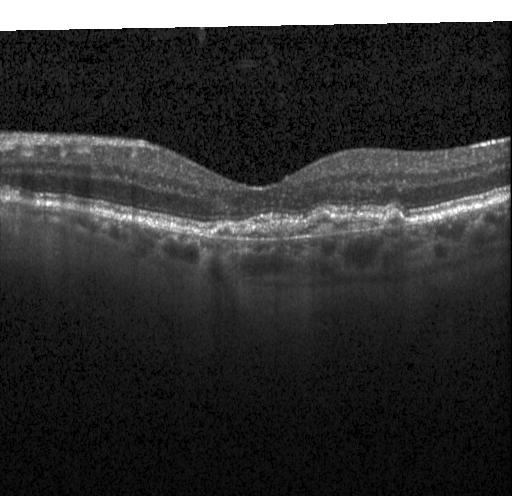 Diagnosis: choroidal neovascularization (CNV).